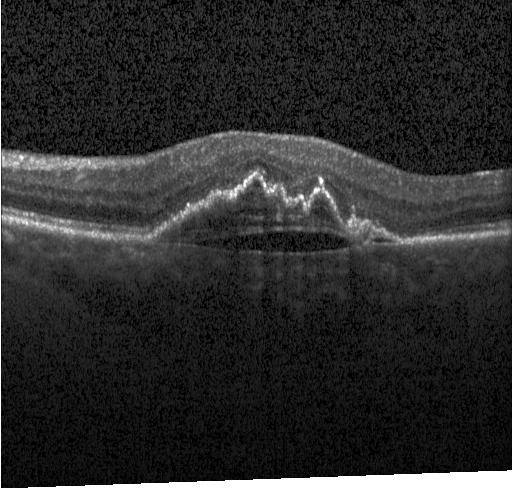
Optical coherence tomography scan · Heidelberg Spectralis OCT system · spectral-domain optical coherence tomography.
Finding: a choroidal neovascular membrane.